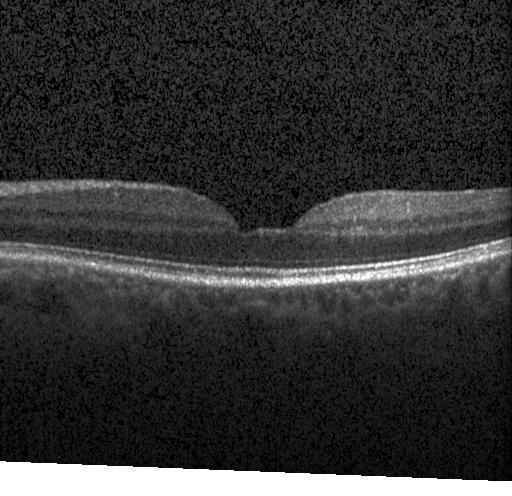

Heidelberg Spectralis, optical coherence tomography scan, centered on the fovea.
Assessment: no CNV, DME, or drusen.